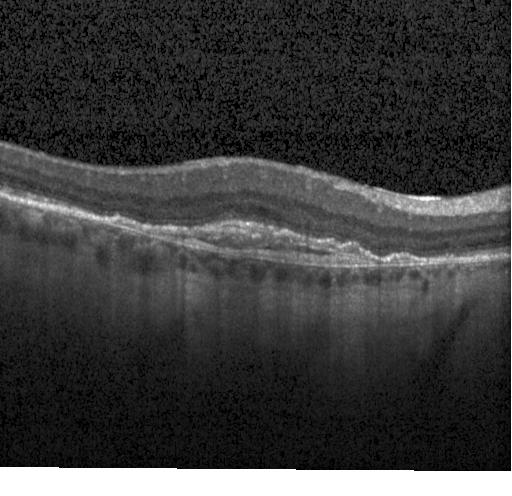 OCT B-scan showing CNV.